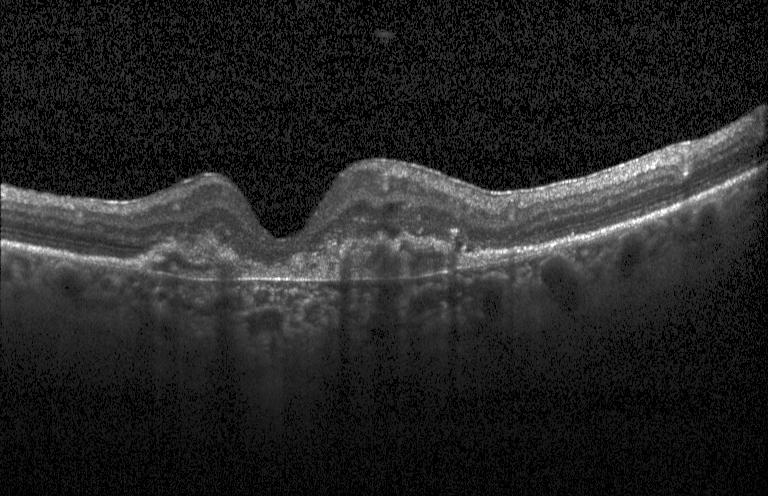

OCT B-scan showing a choroidal neovascular membrane.